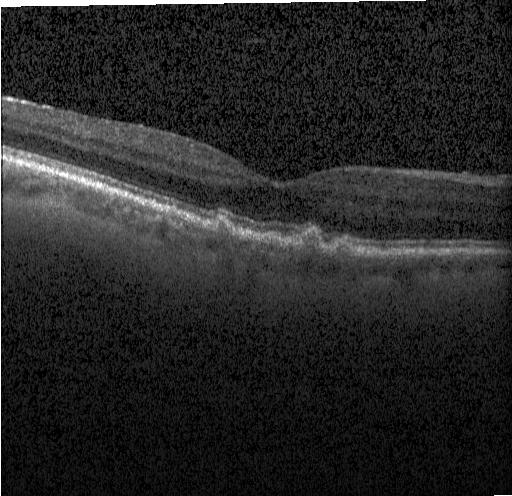
Spectral-domain optical coherence tomography · OCT line scan · fovea-centered · Heidelberg Spectralis OCT system.
Dx: sub-RPE drusenoid deposits.